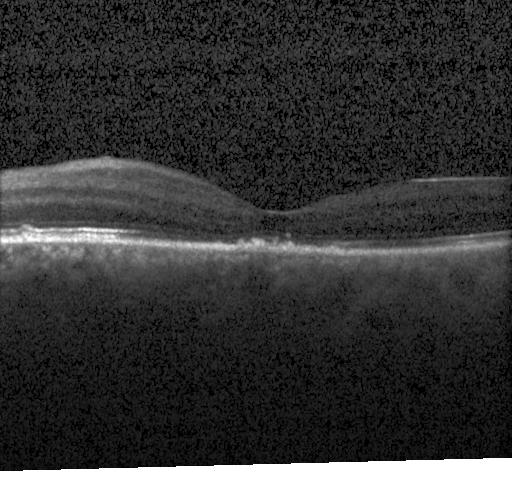

Heidelberg Spectralis OCT system; spectral-domain OCT; retinal OCT cross-section. The scan shows drusen.